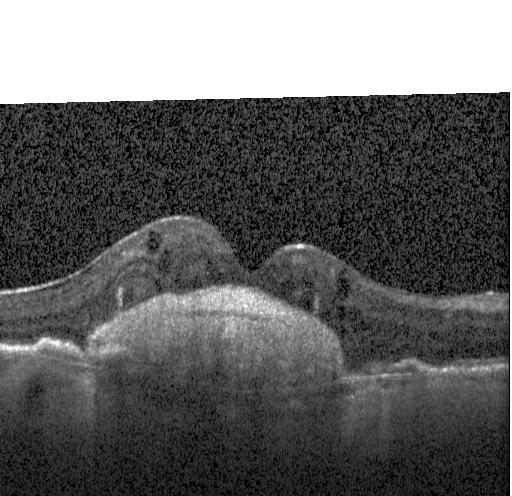 Heidelberg Spectralis OCT system · optical coherence tomography scan · centered on the fovea · SD-OCT.
Finding: choroidal neovascularization.